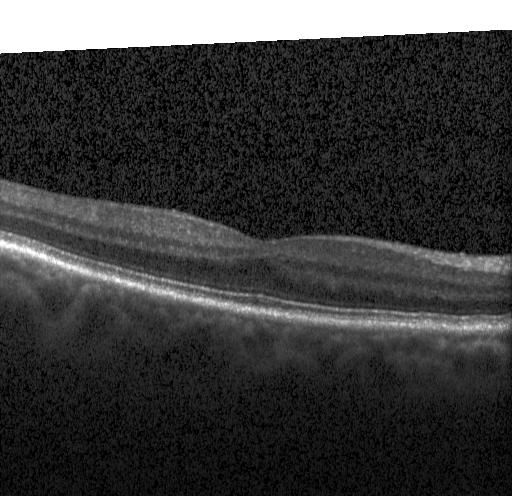

Spectral-domain OCT · Heidelberg Spectralis · optical coherence tomography scan
Neither choroidal neovascularization, diabetic macular edema, nor drusen.